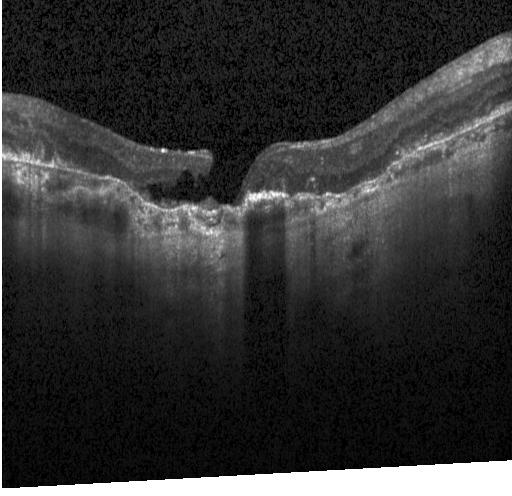
Diagnosis: choroidal neovascularization.